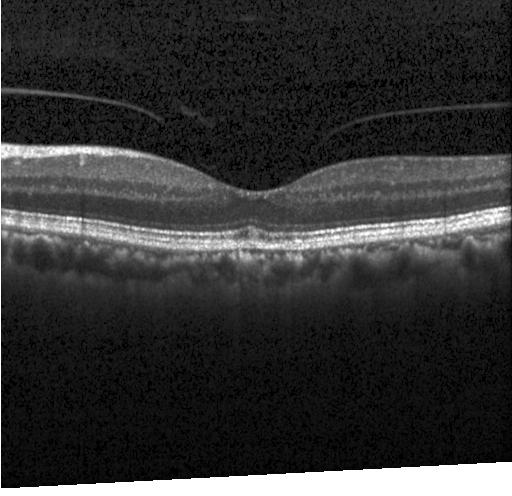

Spectral-domain optical coherence tomography. OCT B-scan
Dx: no CNV, no DME, and no drusen.